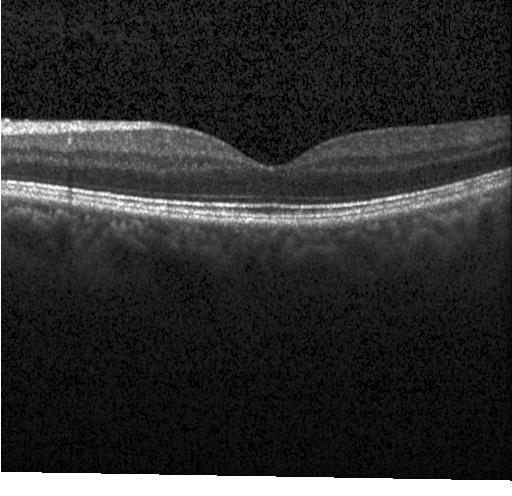
Retinal OCT B-scan.
The scan shows no choroidal neovascularization, no diabetic macular edema, and no drusen.